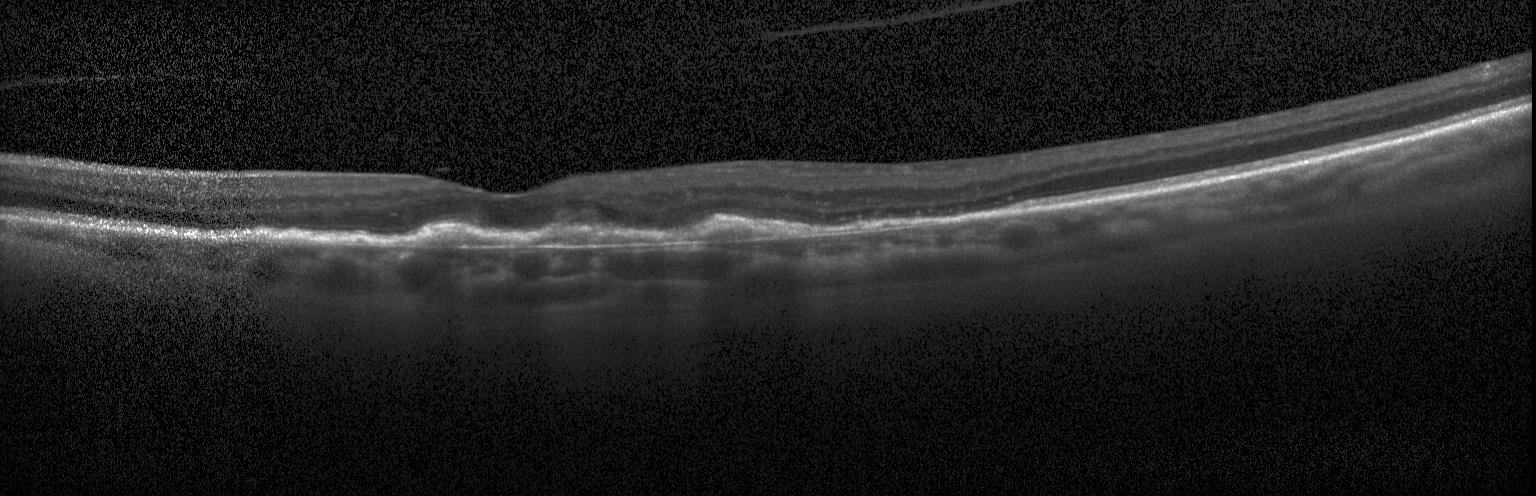
Retinal OCT B-scan · horizontal scan through the fovea · spectral-domain optical coherence tomography — Diagnosis: choroidal neovascularization.